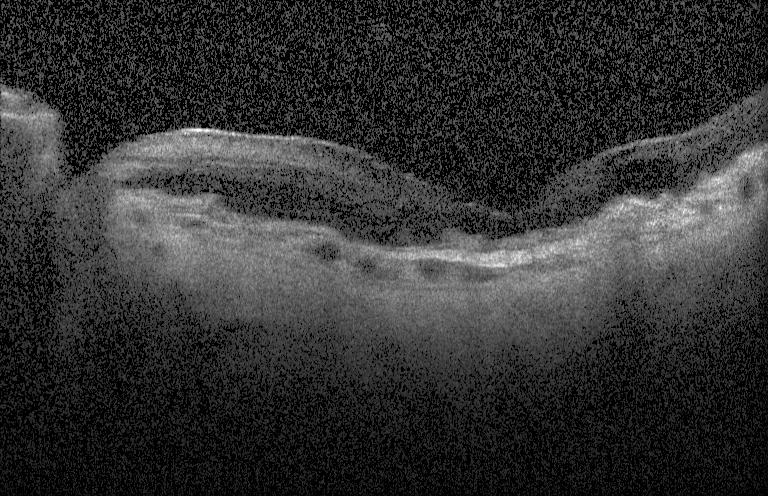 Optical coherence tomography scan · Heidelberg Spectralis — Finding: a choroidal neovascular membrane.